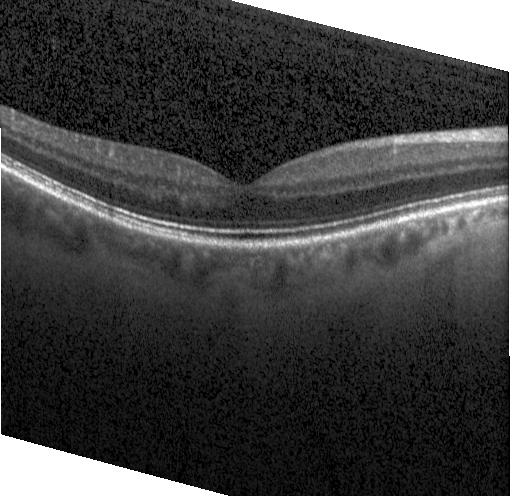
Optical coherence tomography B-scan, through the macula.
OCT finding: no CNV, no DME, and no drusen.